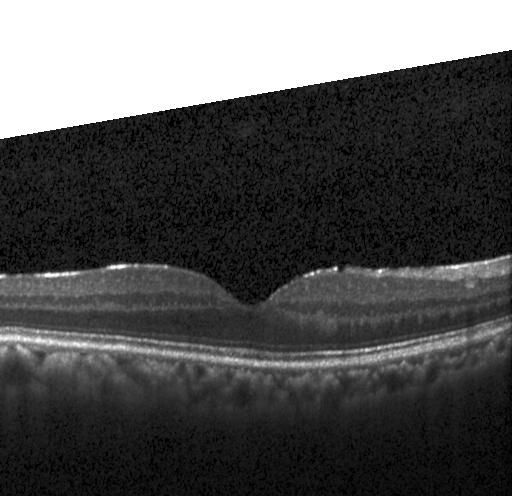

Impression: no choroidal neovascularization, no diabetic macular edema, and no drusen.